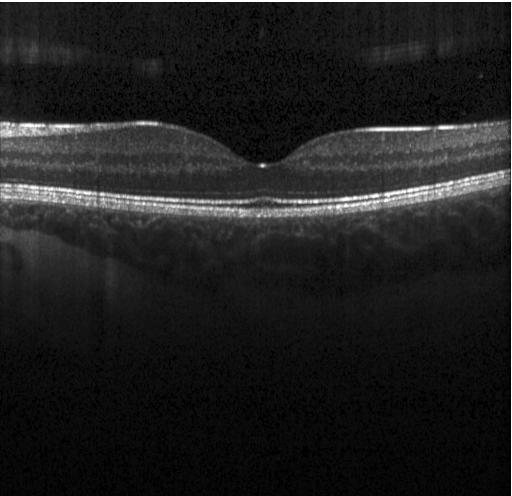
Horizontal scan through the fovea. Optical coherence tomography scan. SD-OCT. Acquired on a Heidelberg Spectralis. Impression: no evidence of choroidal neovascularization, diabetic macular edema, or drusen.